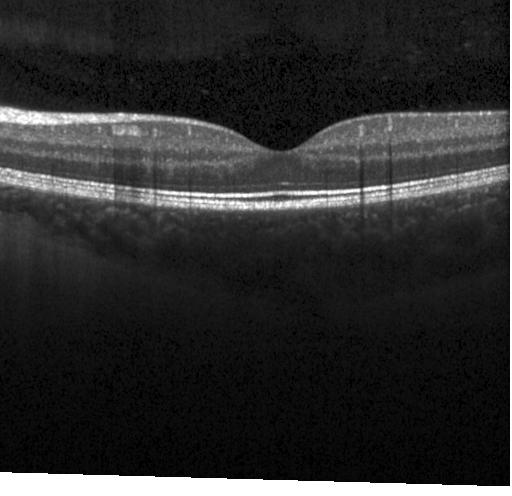 The scan shows no CNV, DME, or drusen.